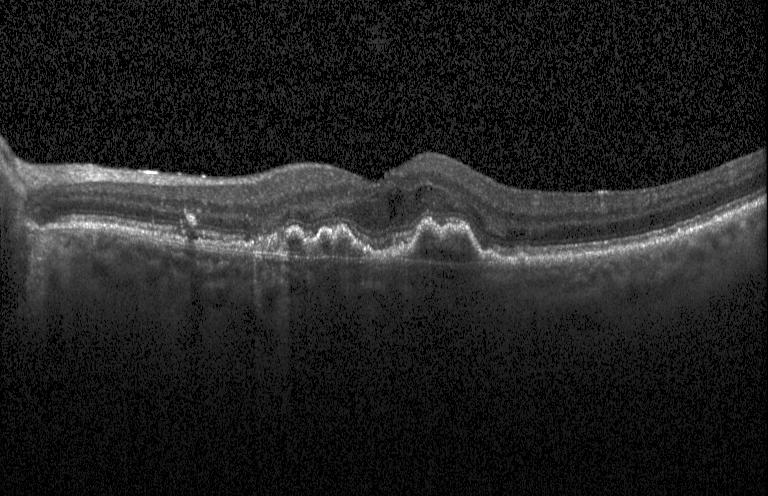

Impression: a choroidal neovascular membrane.